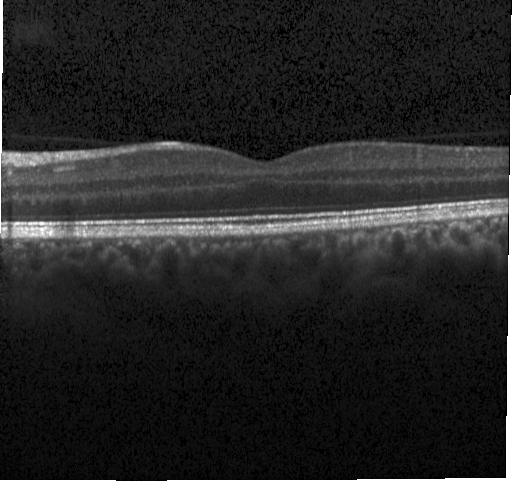 Impression: no evidence of CNV, DME, or drusen.